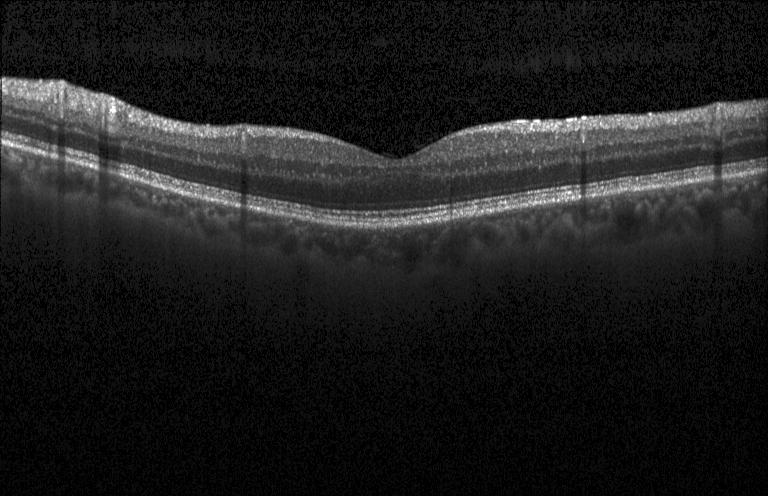
Horizontal scan through the fovea. SD-OCT. Heidelberg Spectralis. OCT B-scan
OCT finding: no evidence of CNV, DME, or drusen.